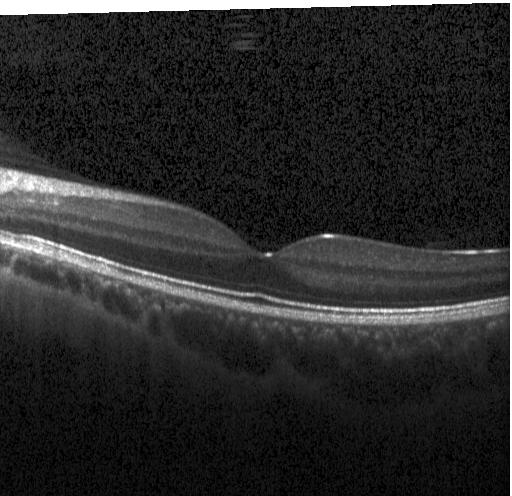

Horizontal scan through the fovea, instrument: Heidelberg Spectralis, OCT B-scan.
This B-scan demonstrates no evidence of CNV, DME, or drusen.